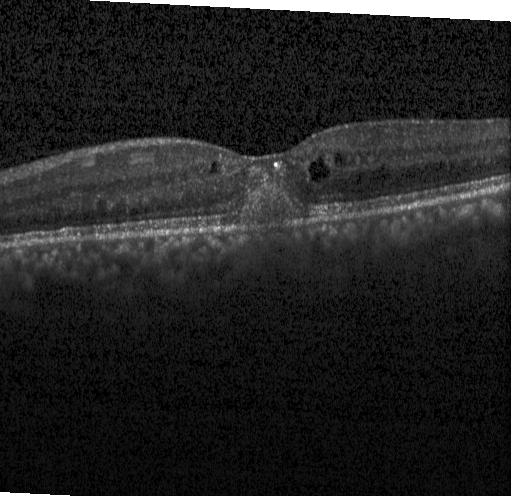 OCT B-scan showing choroidal neovascularization (CNV).